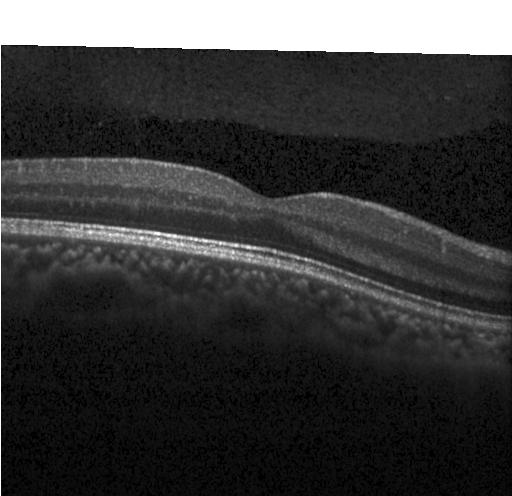
Retinal OCT cross-section showing no CNV, no DME, and no drusen.